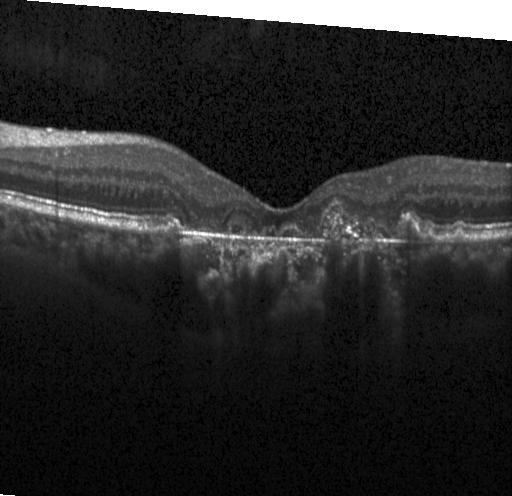

Optical coherence tomography B-scan
Finding: a choroidal neovascular membrane.